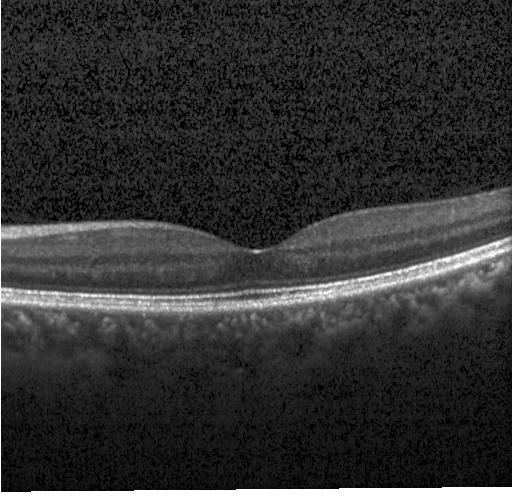

Centered on the fovea; spectral-domain OCT; optical coherence tomography B-scan
Finding: no choroidal neovascularization, no diabetic macular edema, and no drusen.